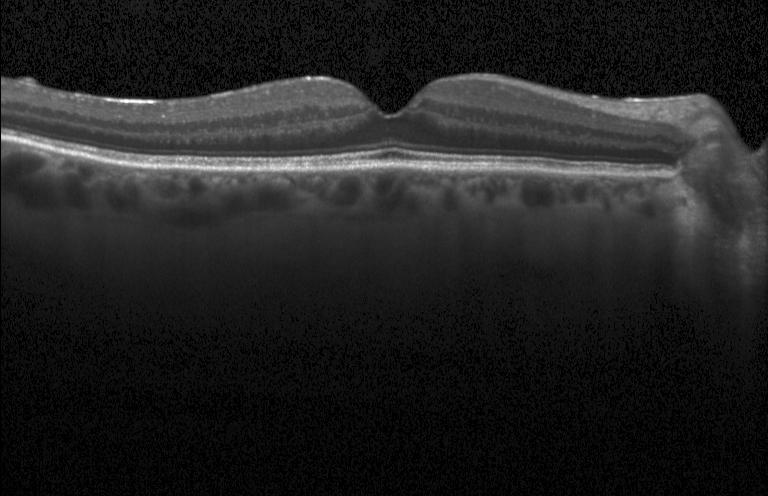 Optical coherence tomography B-scan. This B-scan demonstrates no choroidal neovascularization, diabetic macular edema, or drusen.